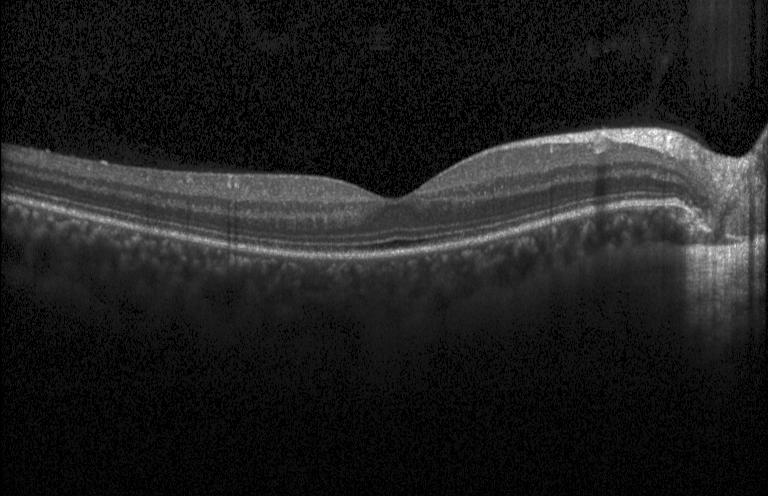 Finding: no evidence of choroidal neovascularization, diabetic macular edema, or drusen.